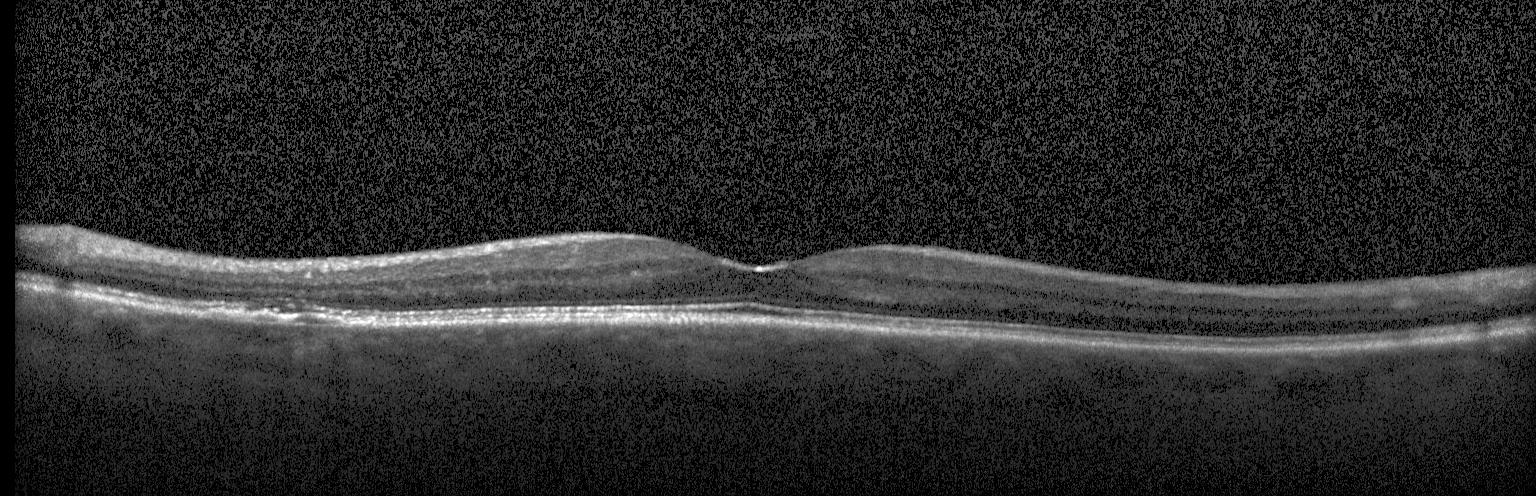
Through the macula. Retinal OCT B-scan.
Dx: a choroidal neovascular membrane.